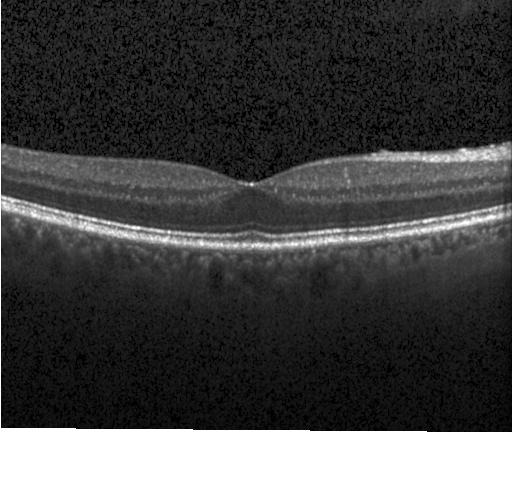
Diagnosis: no choroidal neovascularization, no diabetic macular edema, and no drusen.